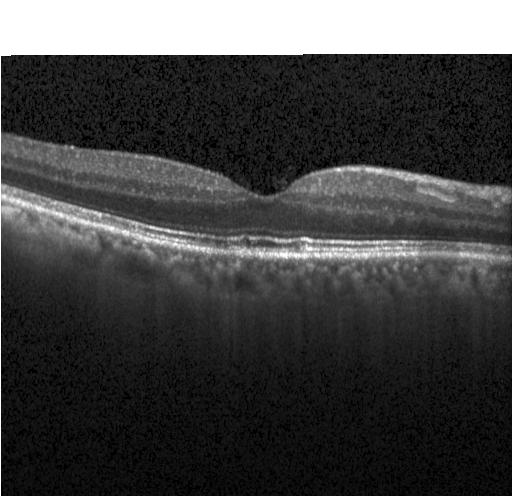

Heidelberg Spectralis OCT system · optical coherence tomography scan · SD-OCT
Macular OCT: no choroidal neovascularization, diabetic macular edema, or drusen.